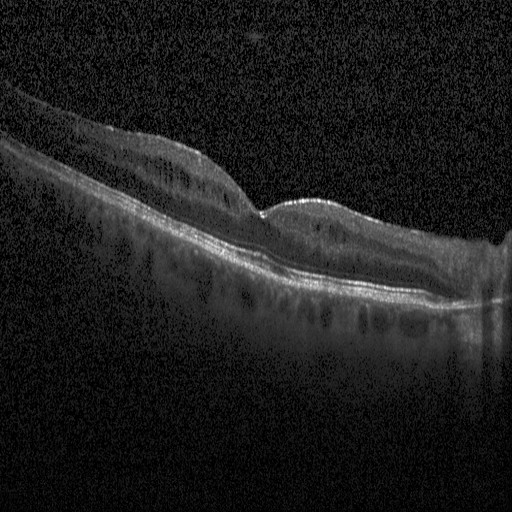
OCT B-scan. Heidelberg Spectralis
Diagnosis: DME.